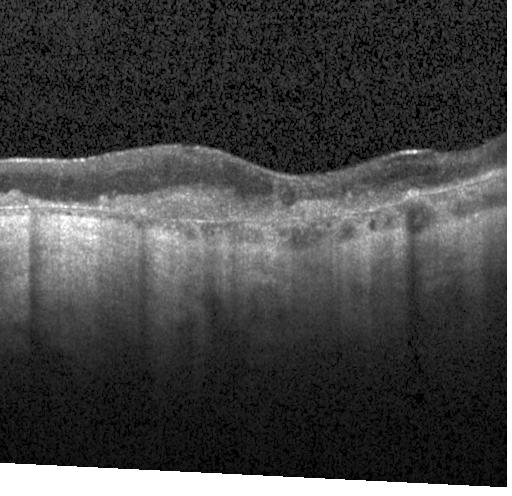 Optical coherence tomography B-scan, acquired on a Heidelberg Spectralis, spectral-domain OCT.
Impression: choroidal neovascularization (CNV).